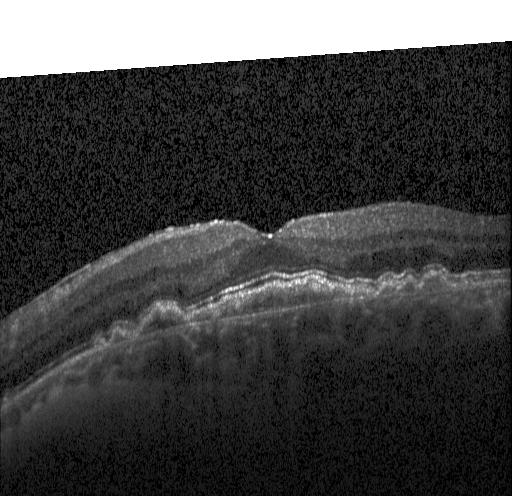
Spectral-domain optical coherence tomography. Horizontal scan through the fovea. Optical coherence tomography B-scan. Heidelberg Spectralis. Finding: CNV.